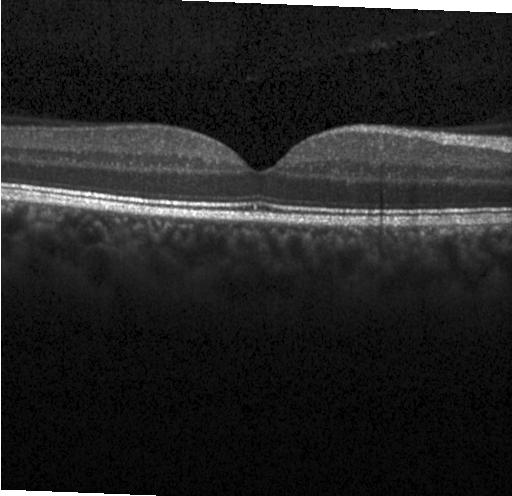
OCT line scan. Horizontal scan through the fovea.
Neither choroidal neovascularization, diabetic macular edema, nor drusen.